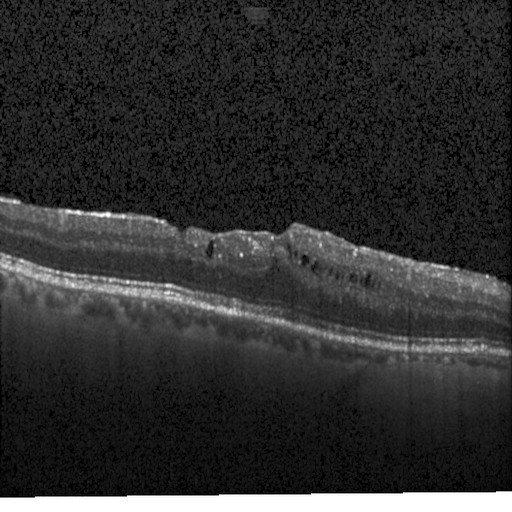 Retinal OCT cross-section. Finding: DME.